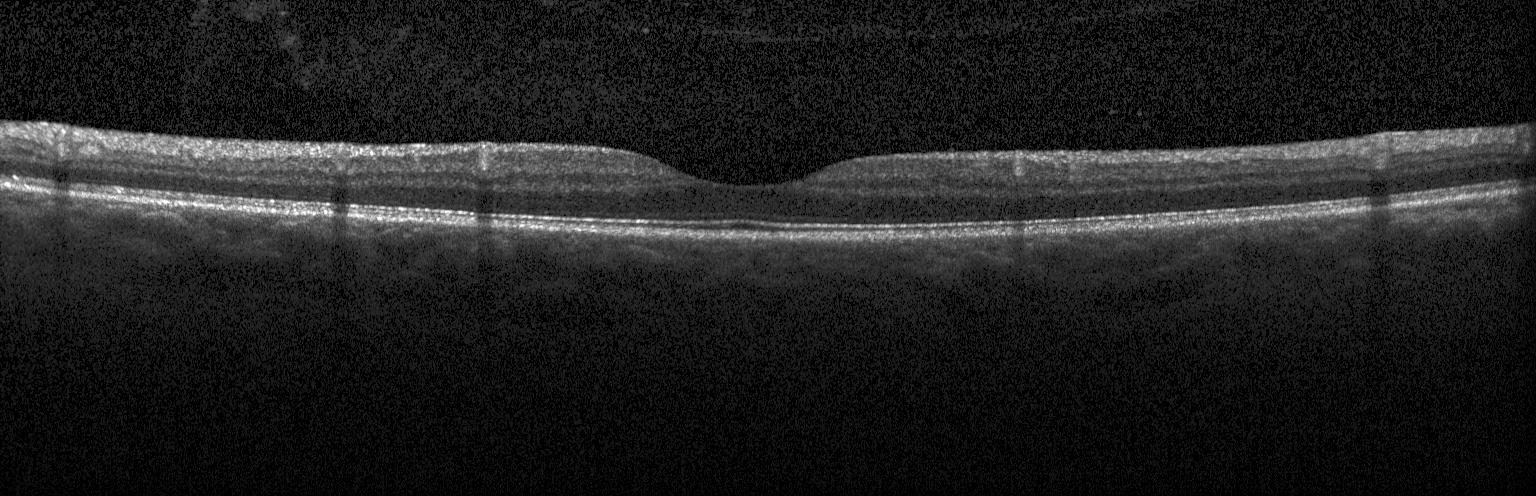 OCT B-scan showing no choroidal neovascularization, diabetic macular edema, or drusen.